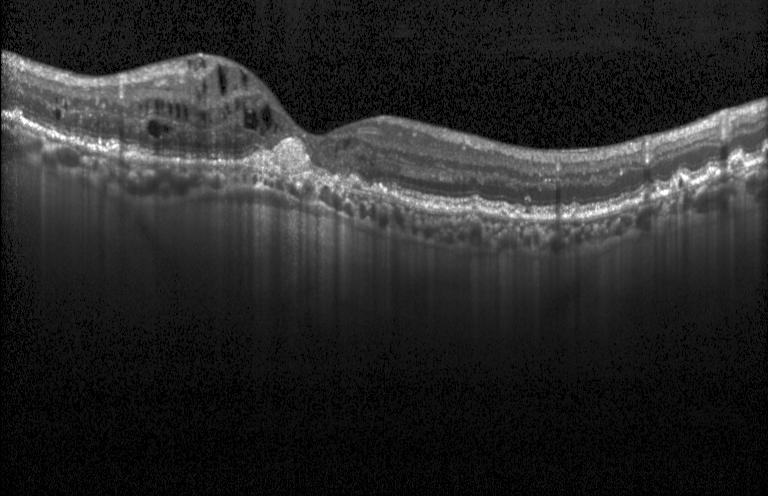
Macular scan; optical coherence tomography B-scan; Heidelberg Spectralis OCT system; spectral-domain optical coherence tomography — Macular OCT: a choroidal neovascular membrane.